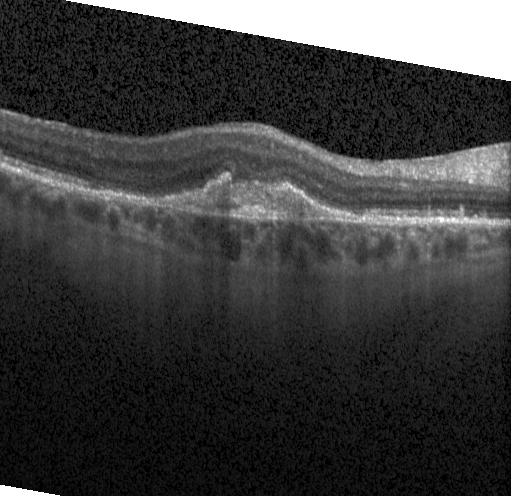
Optical coherence tomography scan · macular scan · Heidelberg Spectralis OCT system · spectral-domain OCT.
CNV.